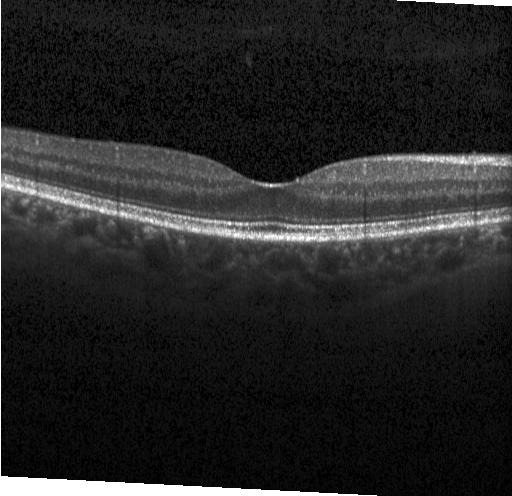
This B-scan demonstrates no CNV, DME, or drusen.